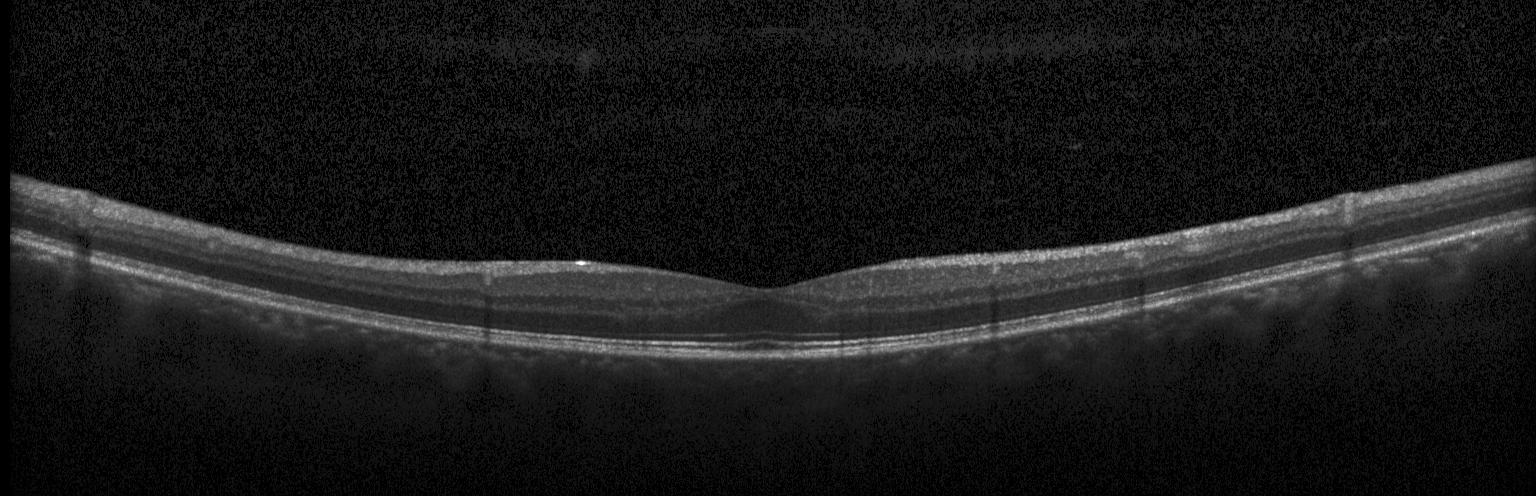
OCT B-scan showing no evidence of choroidal neovascularization, diabetic macular edema, or drusen.